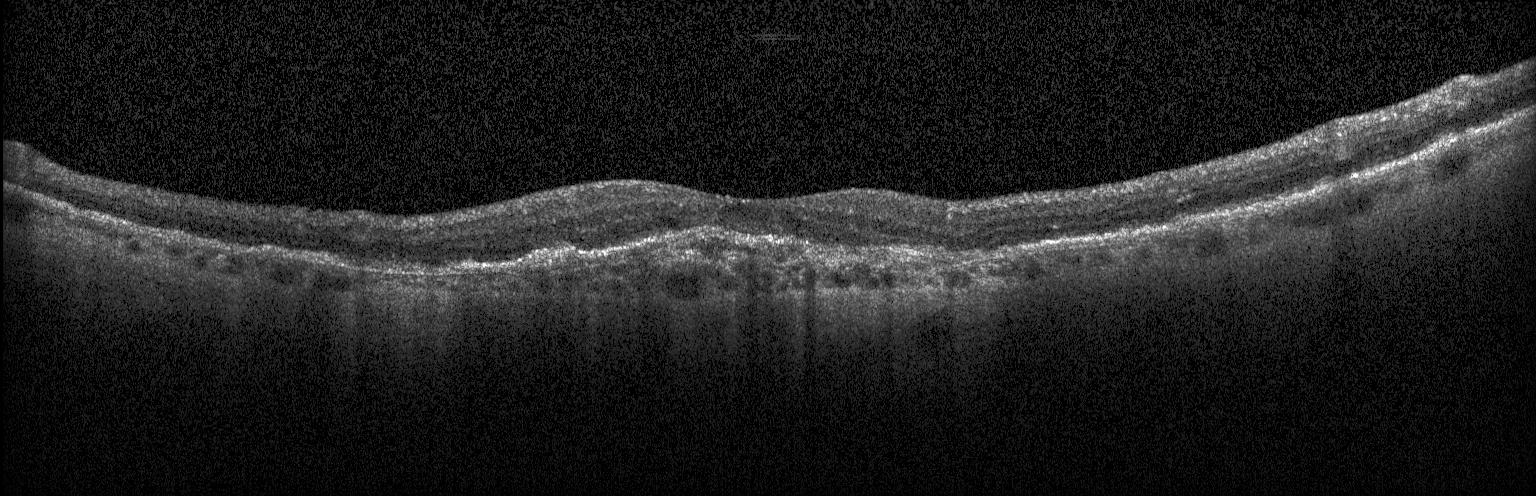

Assessment: a choroidal neovascular membrane.